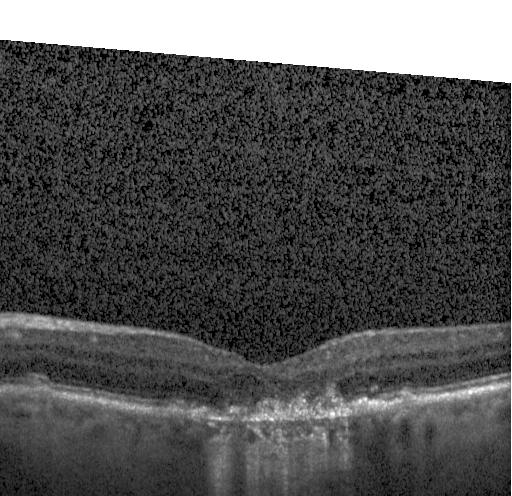

Instrument: Heidelberg Spectralis; OCT B-scan. Finding: CNV.